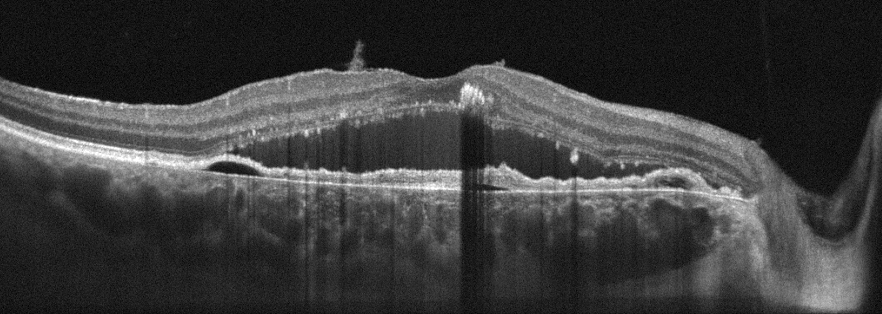 Oculus dexter. OCT B-scan
Assessment: AMD.